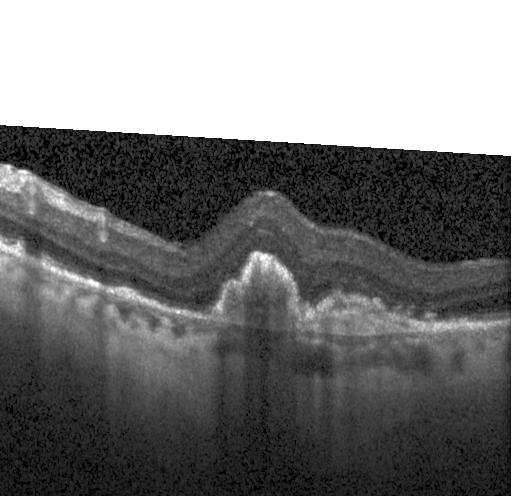

OCT line scan
Finding: CNV.